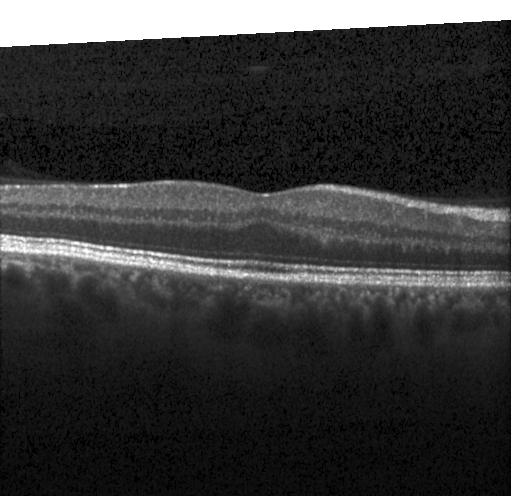

SD-OCT, fovea-centered, acquired on a Heidelberg Spectralis, OCT line scan — No evidence of choroidal neovascularization, diabetic macular edema, or drusen.